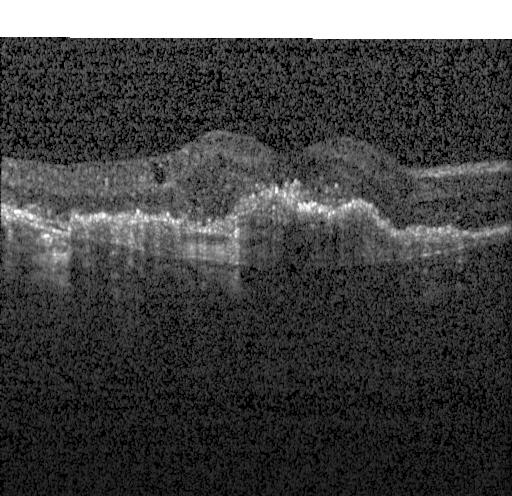 Finding: a choroidal neovascular membrane.